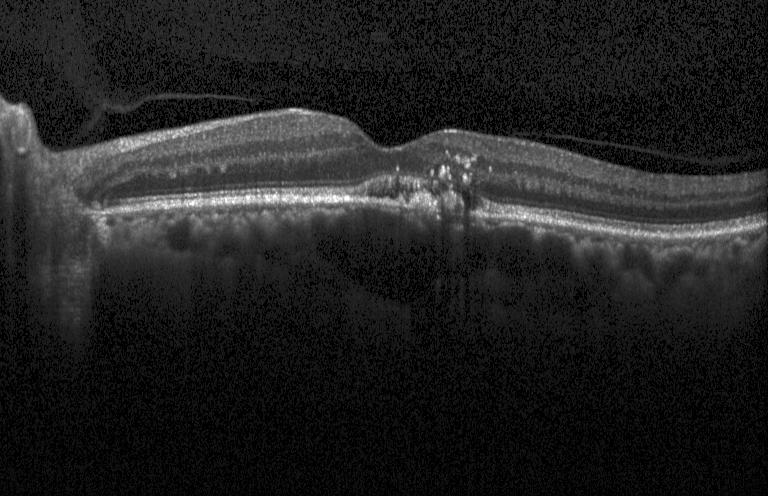

Acquired on a Heidelberg Spectralis. Fovea-centered. SD-OCT. Optical coherence tomography B-scan — Assessment: choroidal neovascularization.